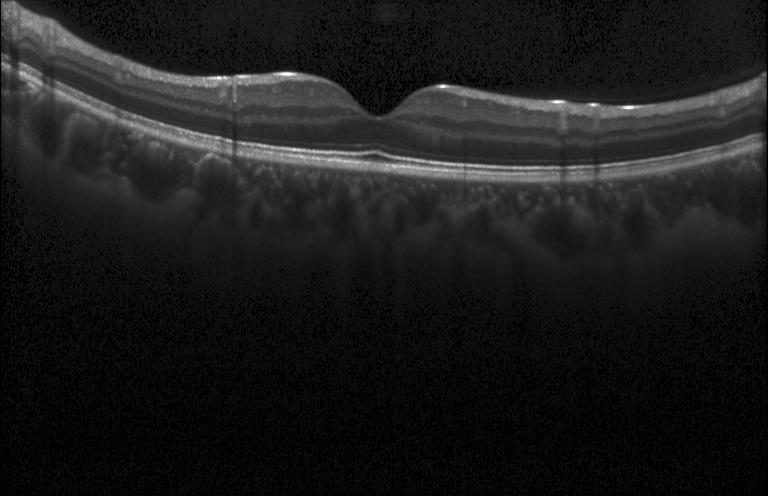
Macular OCT: no CNV, DME, or drusen.